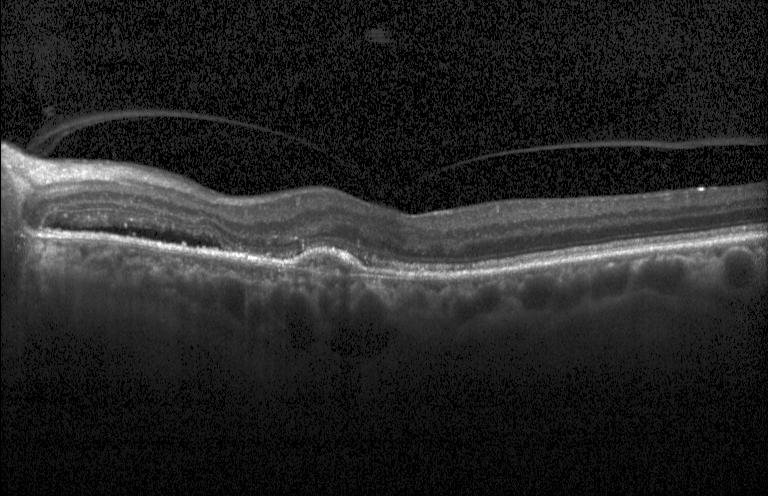
Retinal OCT cross-section.
Diagnosis: a choroidal neovascular membrane.